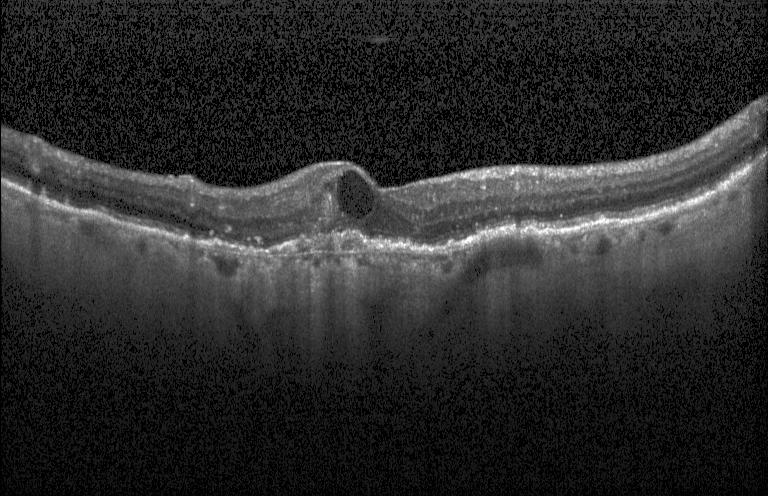
OCT finding: choroidal neovascularization (CNV).